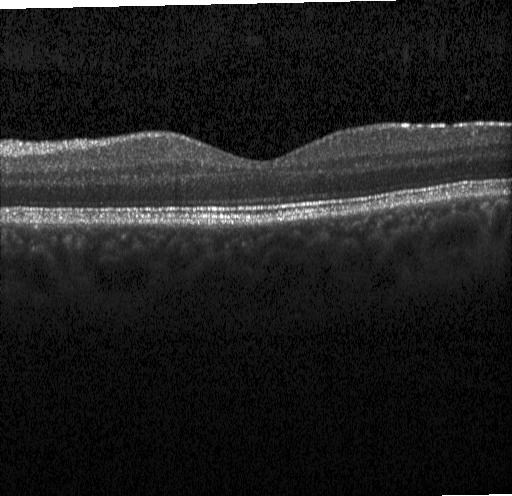 OCT scan showing neither choroidal neovascularization, diabetic macular edema, nor drusen.